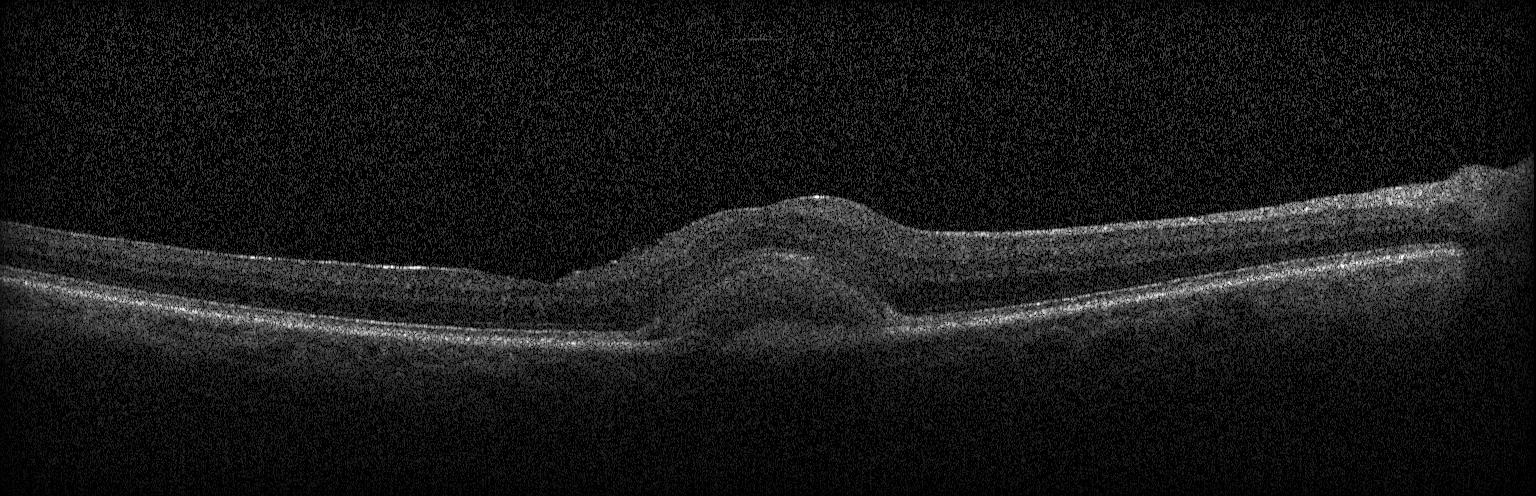
Macular scan. OCT line scan. Heidelberg Spectralis OCT system. Spectral-domain optical coherence tomography.
CNV.